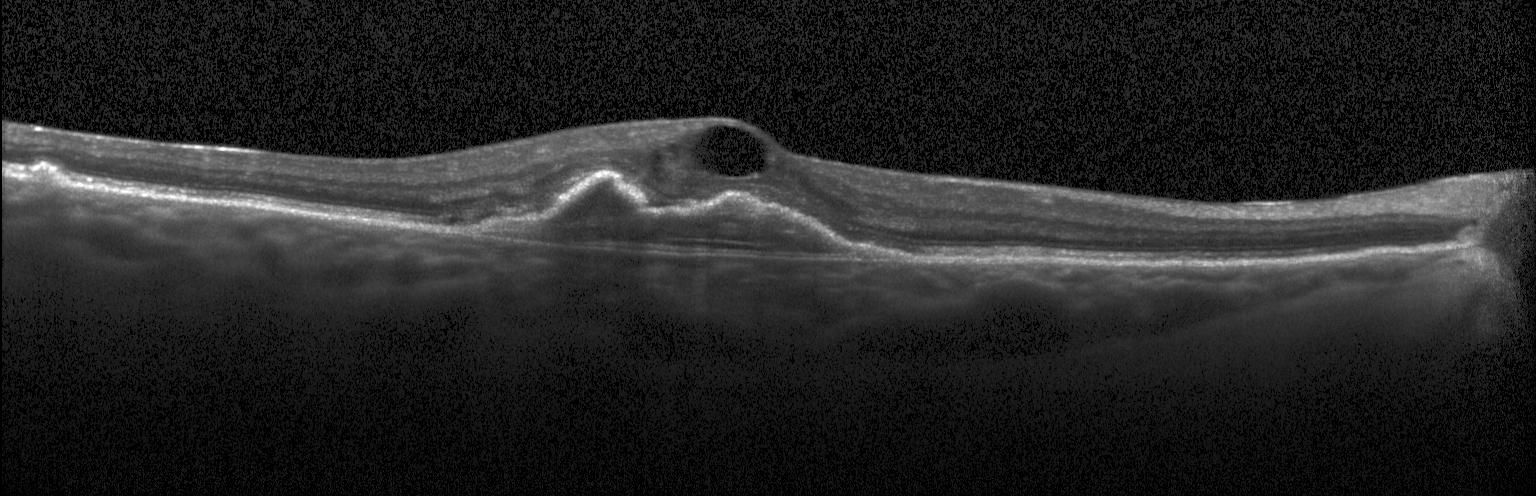

Heidelberg Spectralis OCT system. Retinal OCT cross-section — The scan shows a choroidal neovascular membrane.